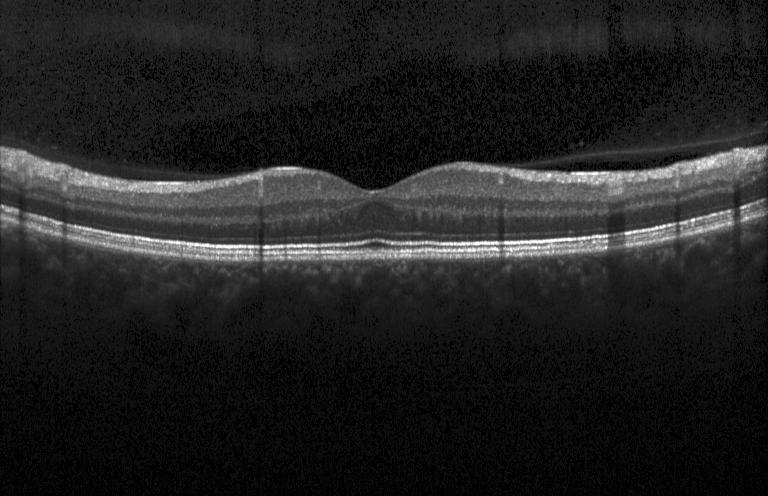
Acquired on a Heidelberg Spectralis; optical coherence tomography scan
Diagnosis: no choroidal neovascularization, diabetic macular edema, or drusen.